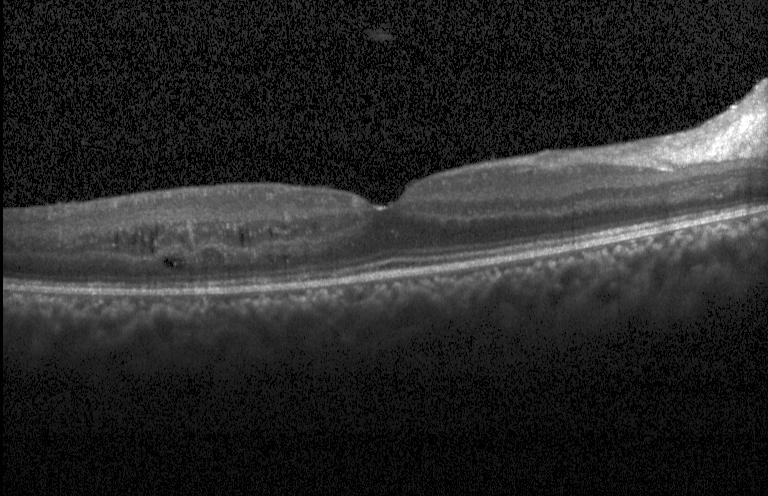

SD-OCT, macular scan, acquired on a Heidelberg Spectralis, OCT B-scan. Diagnosis: diabetic macular edema.